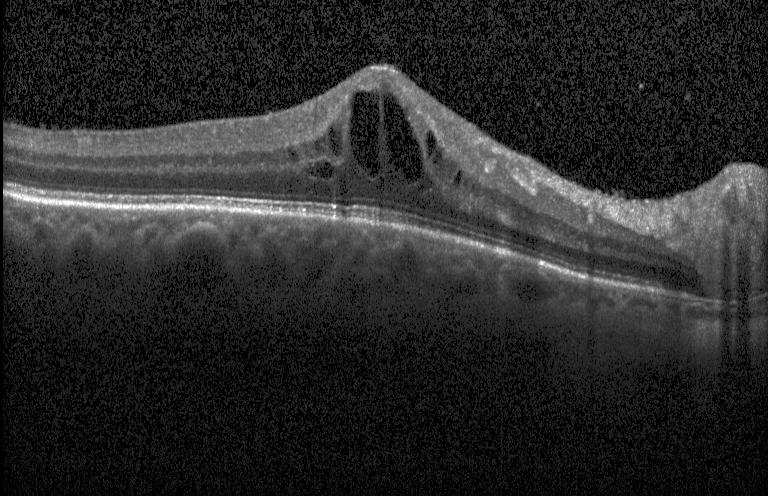

SD-OCT · optical coherence tomography scan · horizontal scan through the fovea · Heidelberg Spectralis OCT system — Finding: DME.